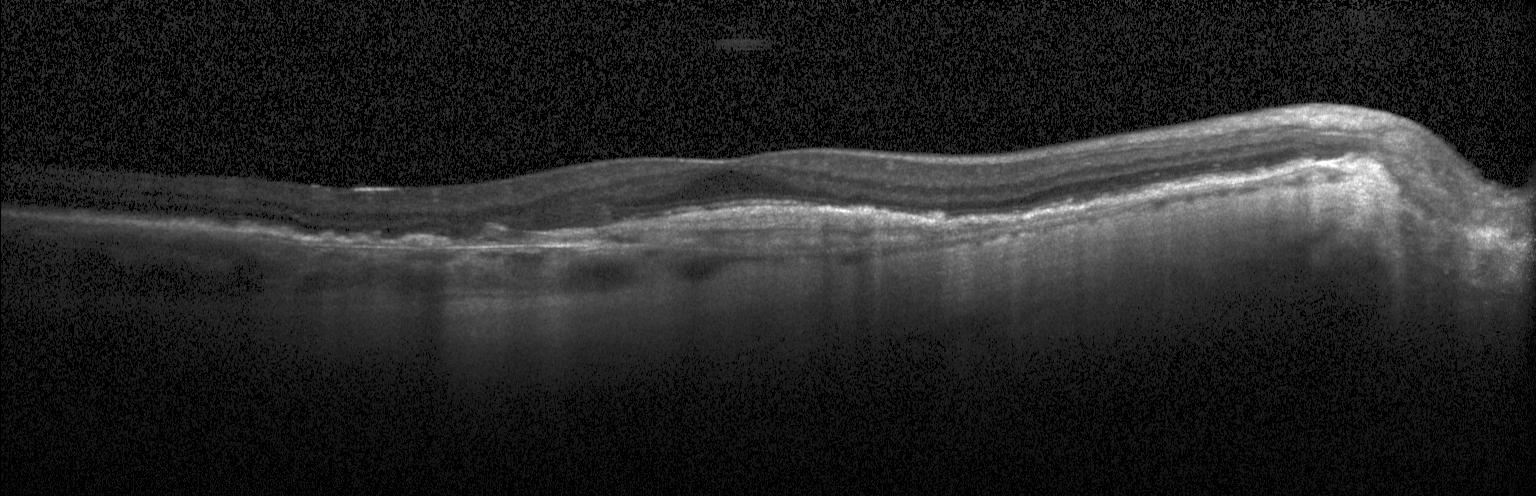
OCT line scan; SD-OCT — This B-scan demonstrates choroidal neovascularization.